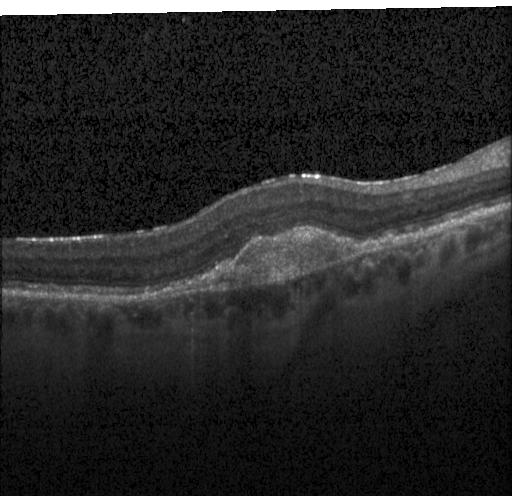
Impression: a choroidal neovascular membrane.